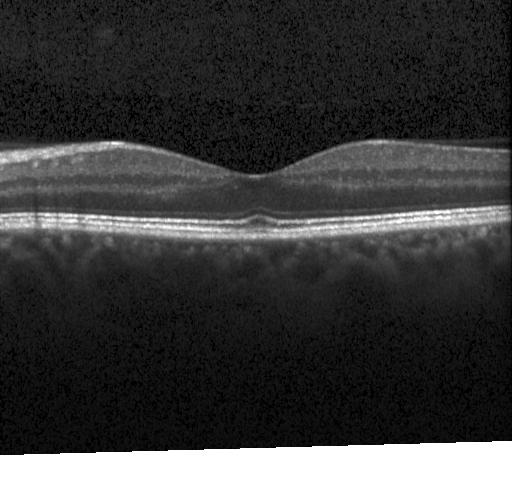
Spectral-domain optical coherence tomography. Optical coherence tomography scan. Heidelberg Spectralis. Assessment: no CNV, no DME, and no drusen.